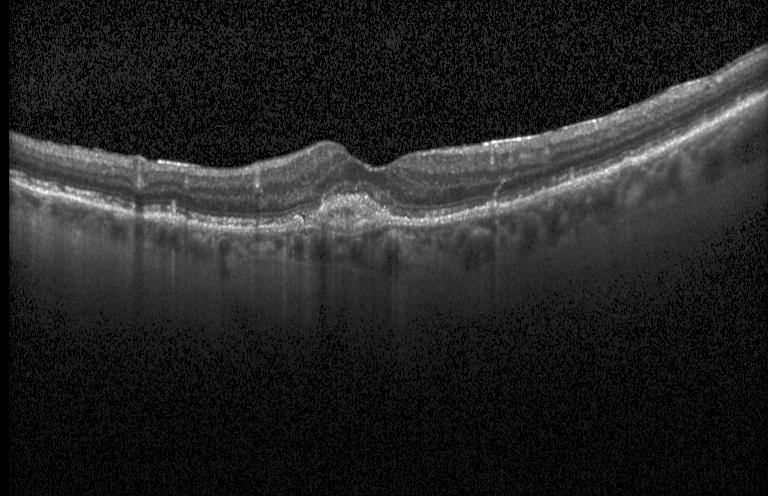

Macular OCT demonstrating a choroidal neovascular membrane.